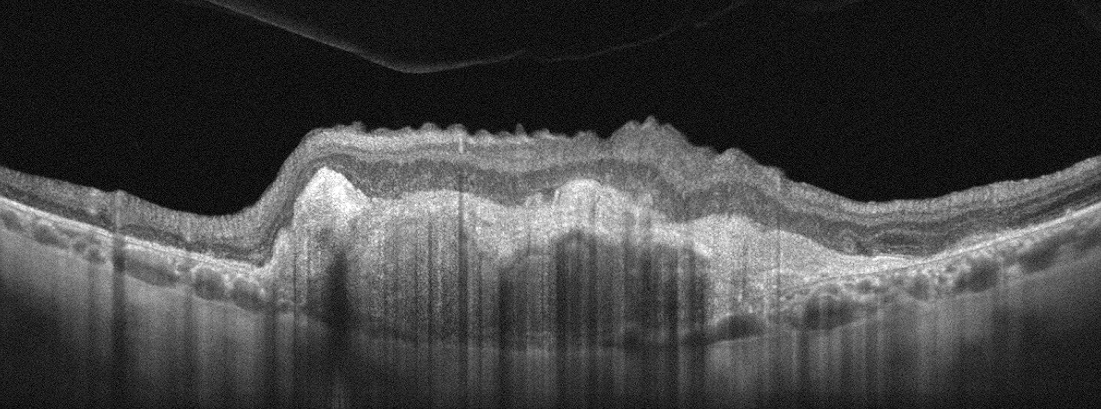

Finding: age-related macular degeneration.